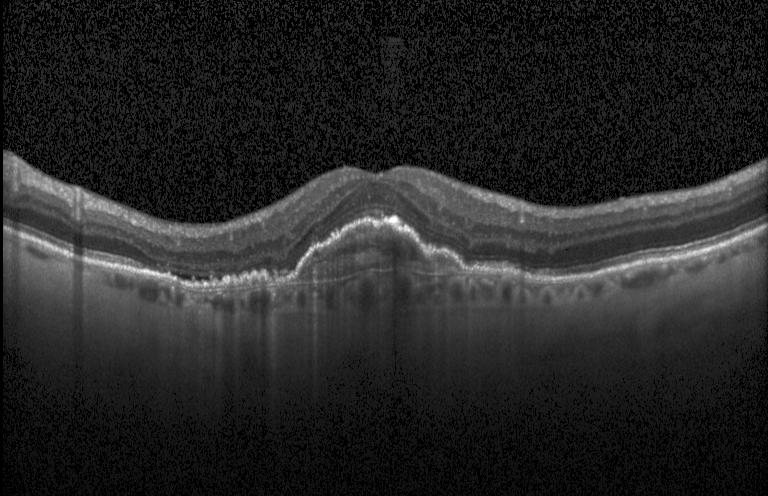

Spectral-domain optical coherence tomography; fovea-centered; acquired on a Heidelberg Spectralis; optical coherence tomography B-scan. Macular OCT: choroidal neovascularization (CNV).